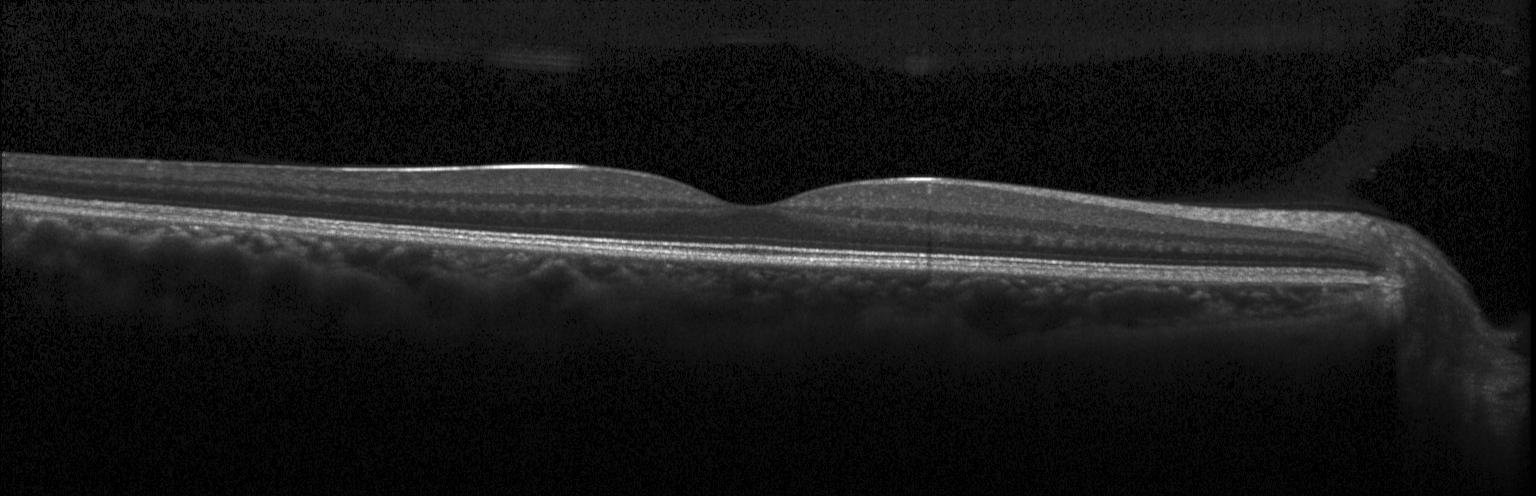 Optical coherence tomography scan, spectral-domain optical coherence tomography.
Diagnosis: no evidence of choroidal neovascularization, diabetic macular edema, or drusen.